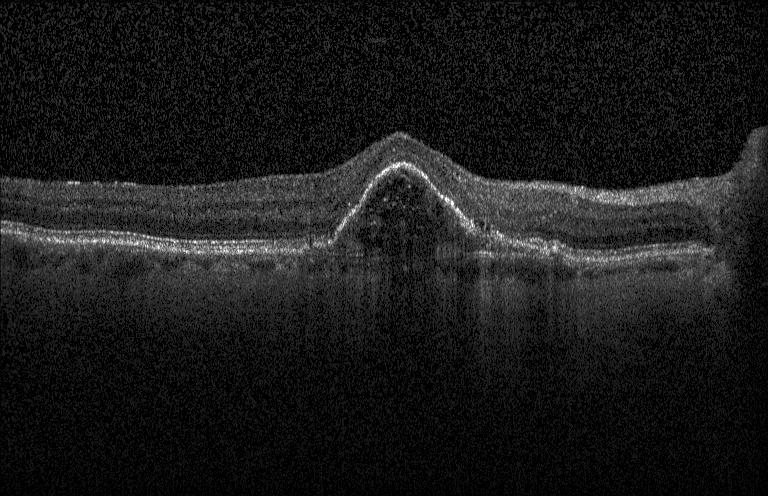
Optical coherence tomography scan — Diagnosis: a choroidal neovascular membrane.